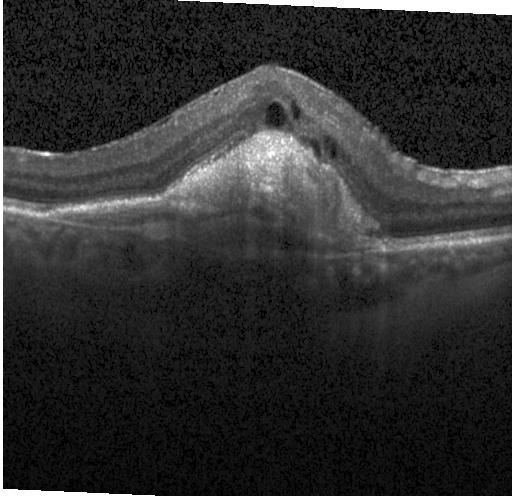 Centered on the fovea. Retinal OCT cross-section. Heidelberg Spectralis. Spectral-domain optical coherence tomography.
Dx: a choroidal neovascular membrane.